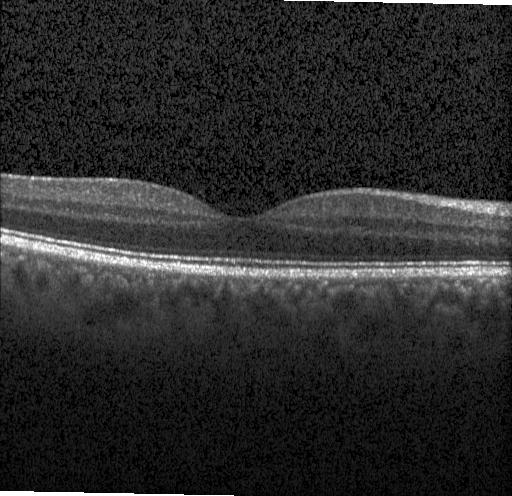

Optical coherence tomography scan. This B-scan demonstrates no choroidal neovascularization, diabetic macular edema, or drusen.